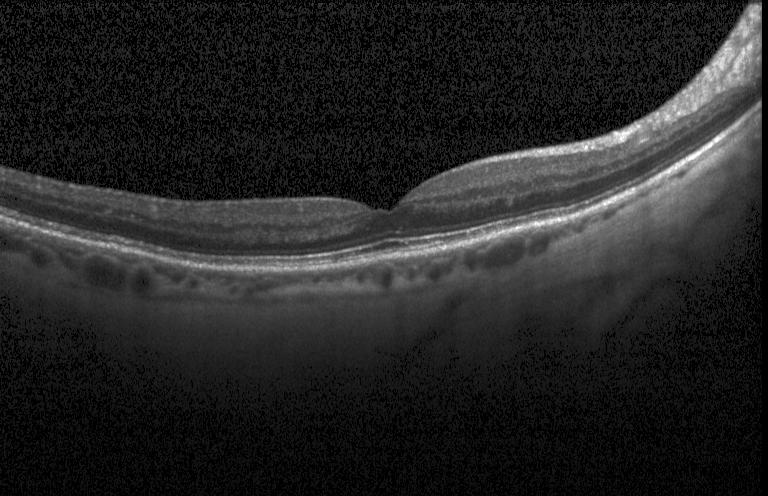 Macular OCT demonstrating no choroidal neovascularization, no diabetic macular edema, and no drusen.